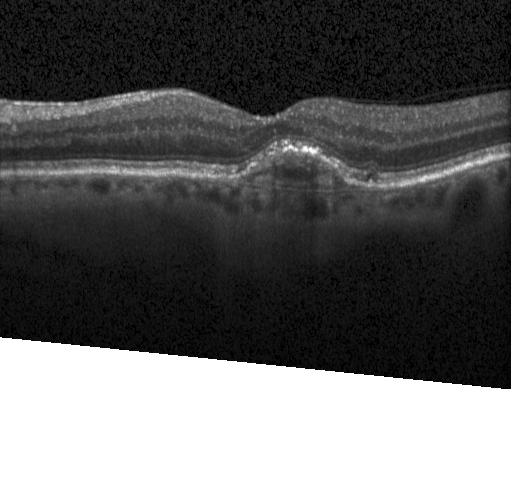

Dx: choroidal neovascularization (CNV).